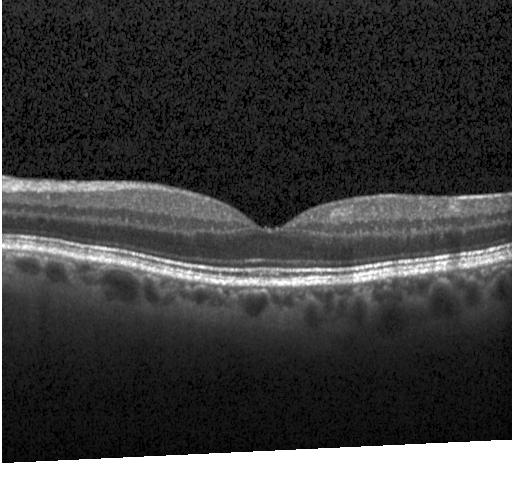

Retinal OCT cross-section
Neither CNV, DME, nor drusen.